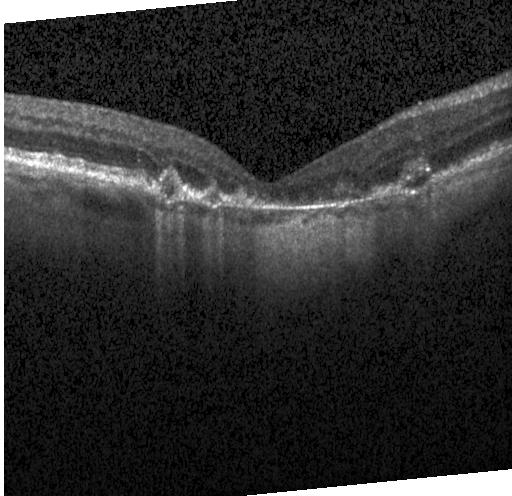
Diagnosis: CNV.